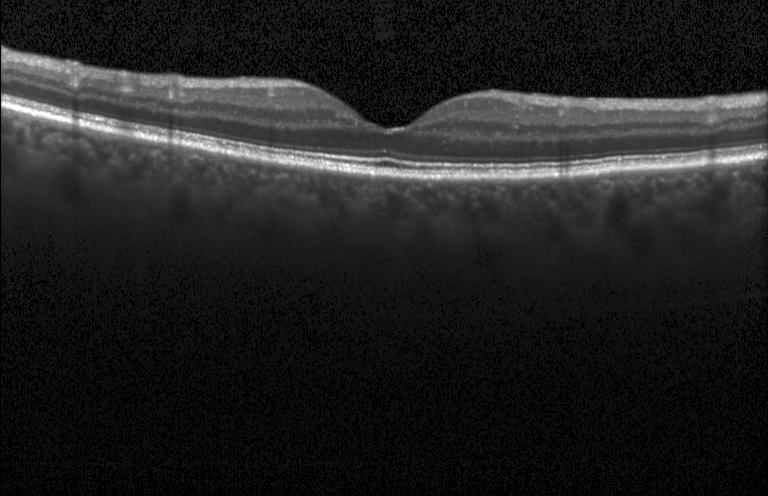 Optical coherence tomography scan — The scan shows no evidence of CNV, DME, or drusen.